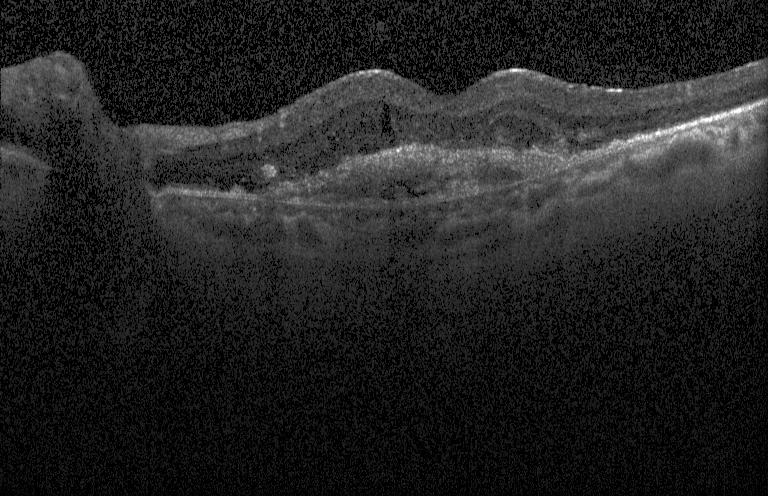 SD-OCT. OCT B-scan. Horizontal scan through the fovea.
Finding: CNV.